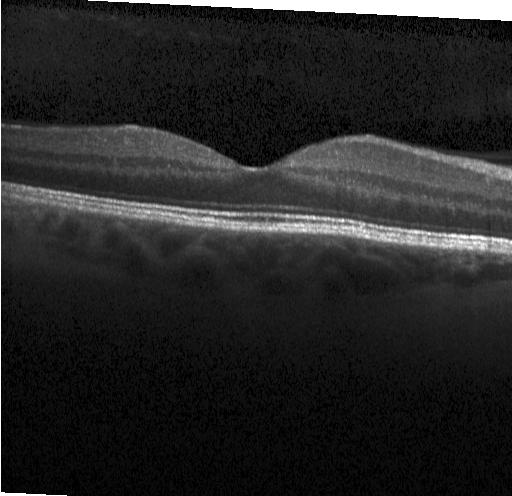 Optical coherence tomography B-scan
OCT finding: no evidence of choroidal neovascularization, diabetic macular edema, or drusen.